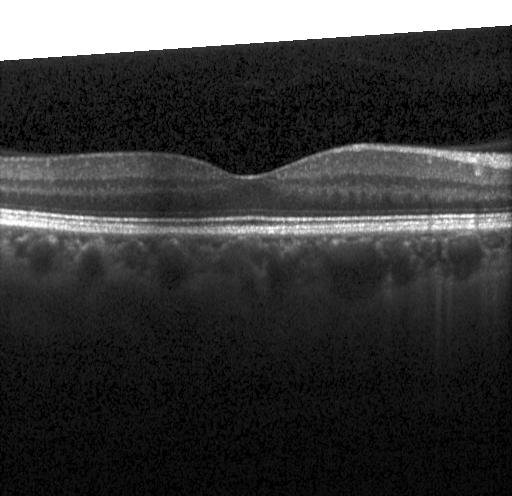 OCT B-scan showing no CNV, no DME, and no drusen.